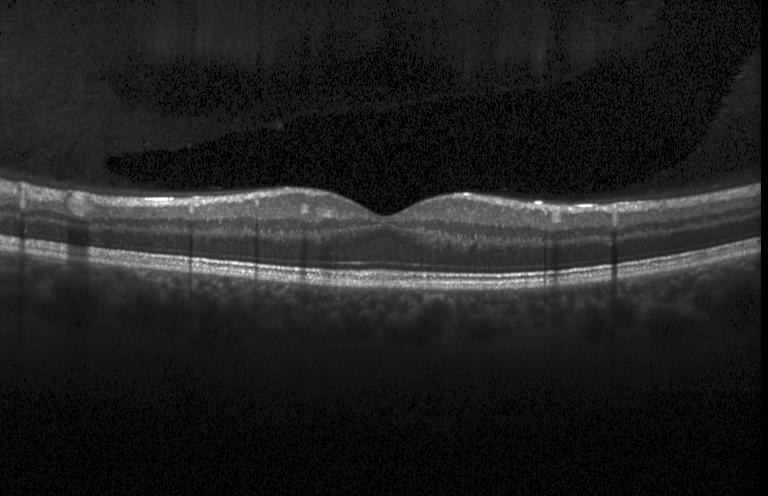
Acquired on a Heidelberg Spectralis; OCT line scan. Finding: no CNV, no DME, and no drusen.